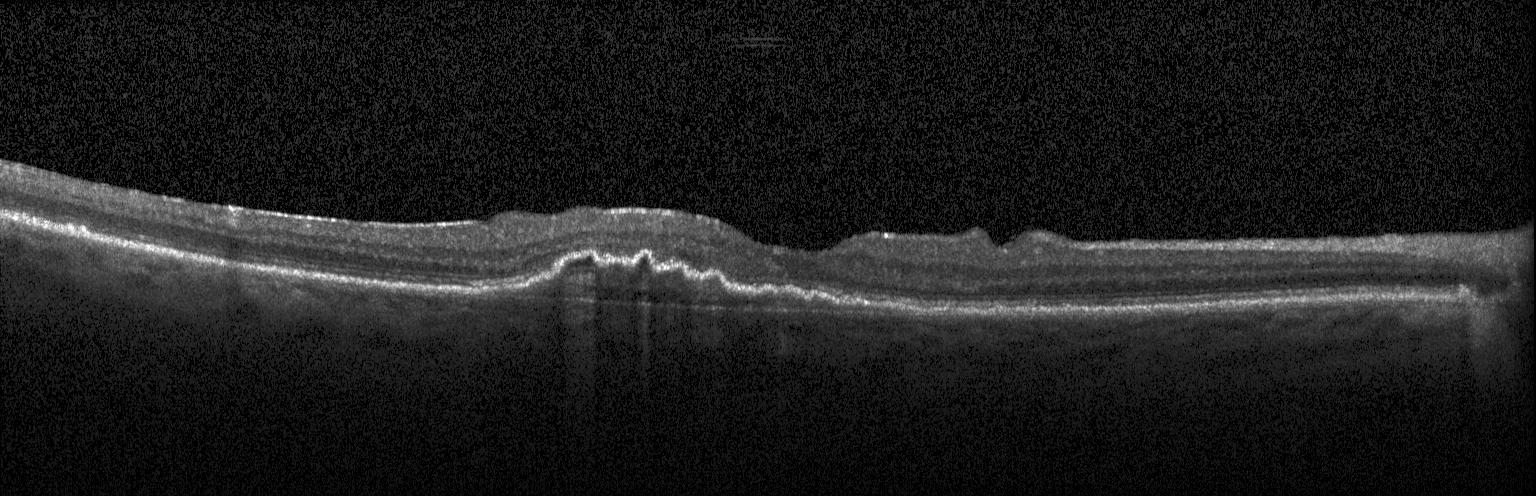

Macular scan; OCT line scan; Heidelberg Spectralis OCT system; SD-OCT
Finding: CNV.